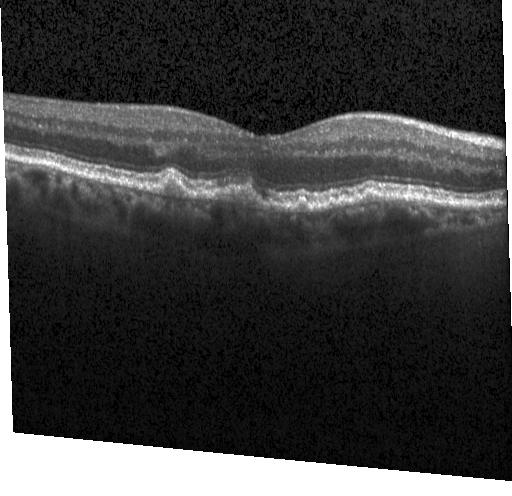

OCT finding: multiple drusen.